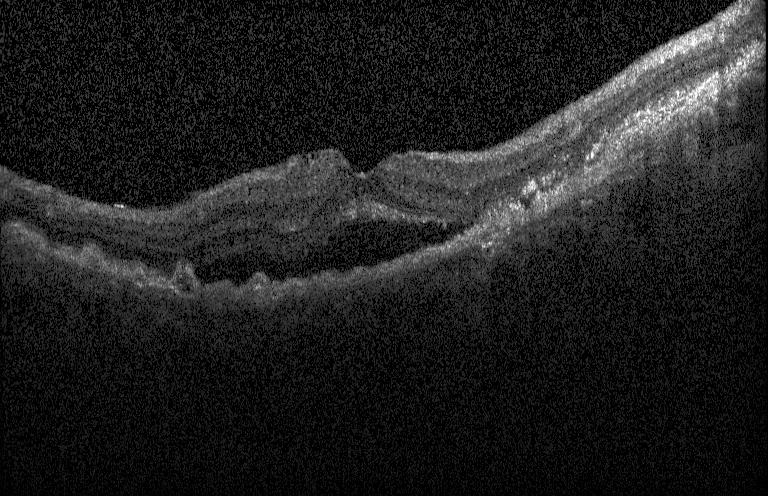
Fovea-centered. Optical coherence tomography scan.
Diagnosis: a choroidal neovascular membrane.